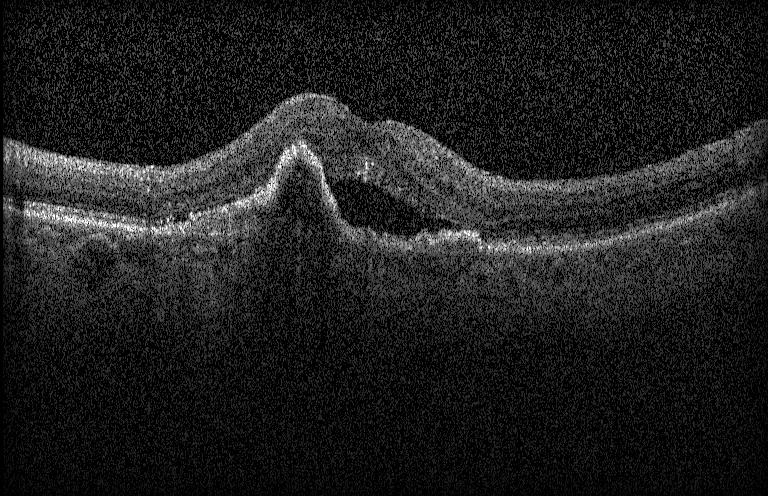 The scan shows CNV.